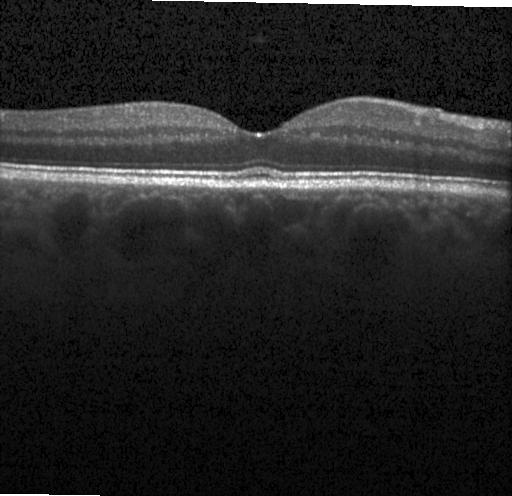
SD-OCT · instrument: Heidelberg Spectralis · retinal OCT cross-section. Finding: no choroidal neovascularization, no diabetic macular edema, and no drusen.